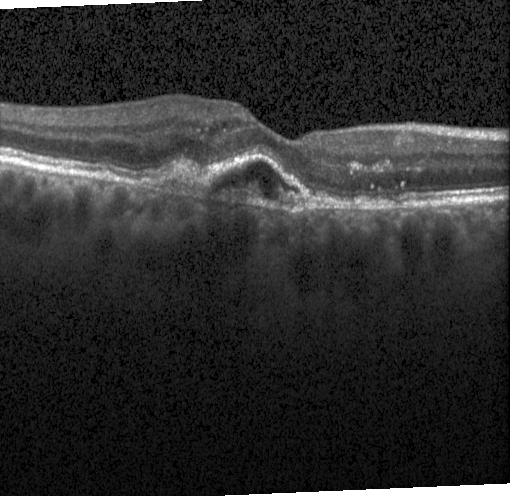 A choroidal neovascular membrane.